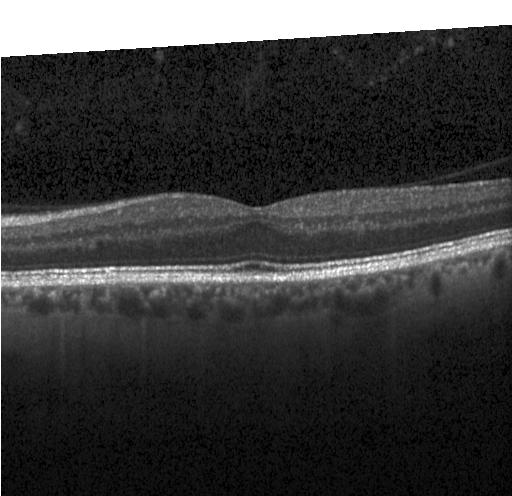 SD-OCT · OCT line scan
The scan shows no CNV, DME, or drusen.